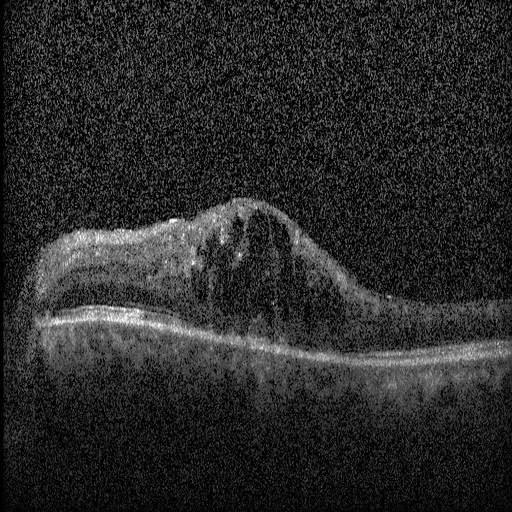 Dx: DME.